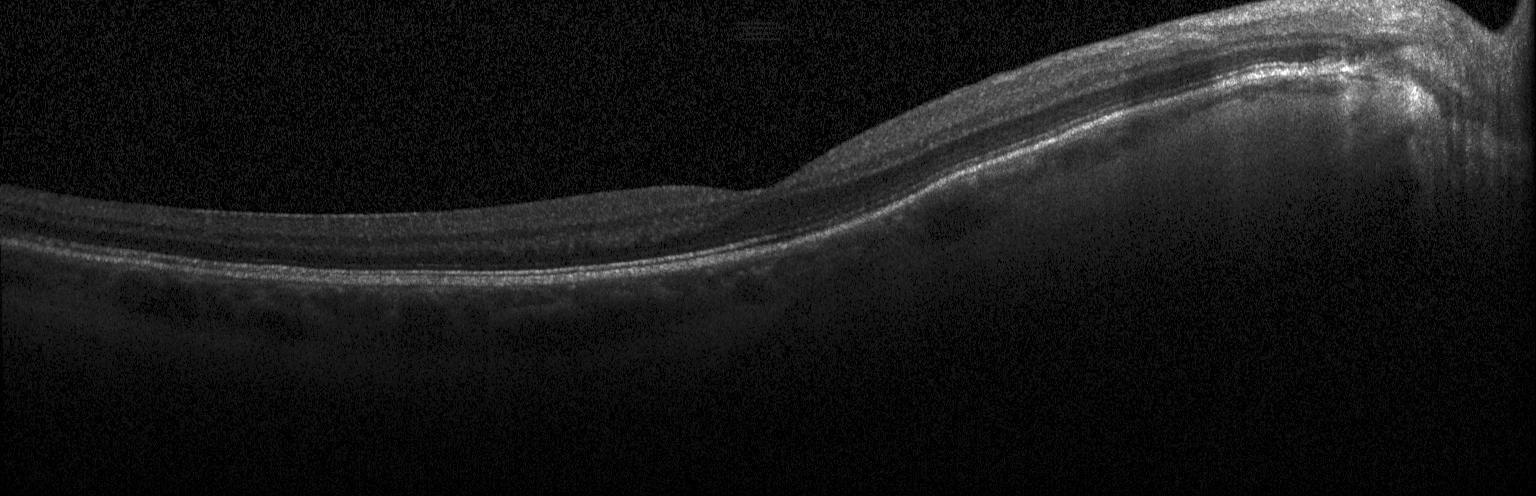

Retinal OCT cross-section
Macular OCT: no evidence of choroidal neovascularization, diabetic macular edema, or drusen.